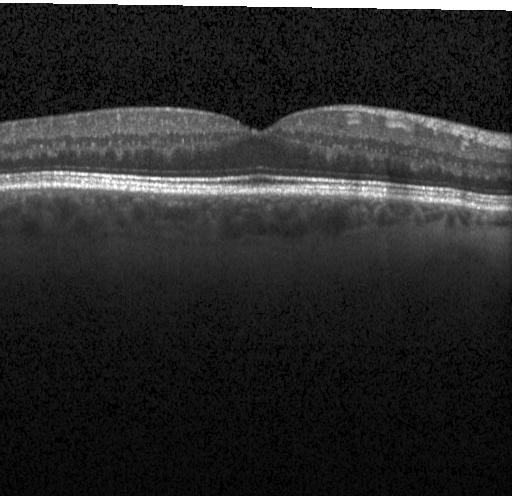 Horizontal scan through the fovea; SD-OCT; optical coherence tomography B-scan.
Assessment: no CNV, no DME, and no drusen.